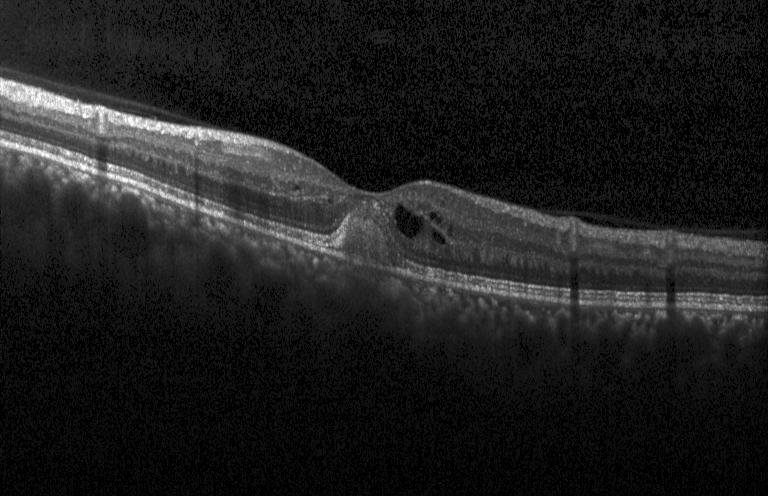 Retinal OCT cross-section showing a choroidal neovascular membrane.